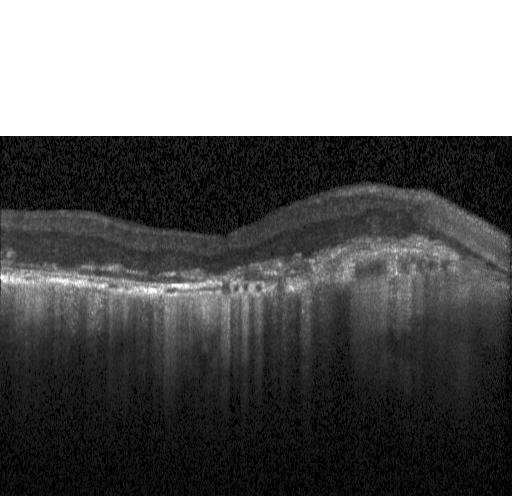

Finding: a choroidal neovascular membrane.